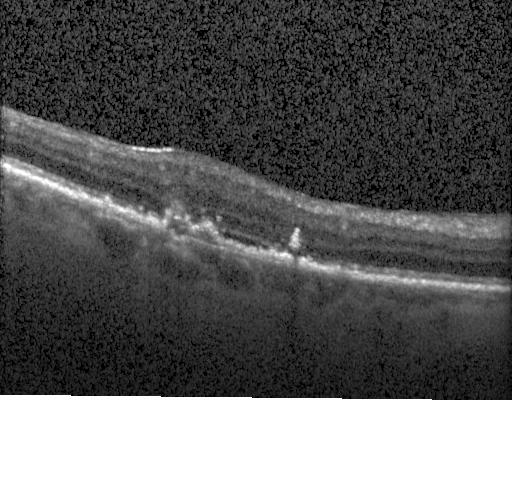

Centered on the fovea. Optical coherence tomography B-scan. Spectral-domain optical coherence tomography — Dx: a choroidal neovascular membrane.